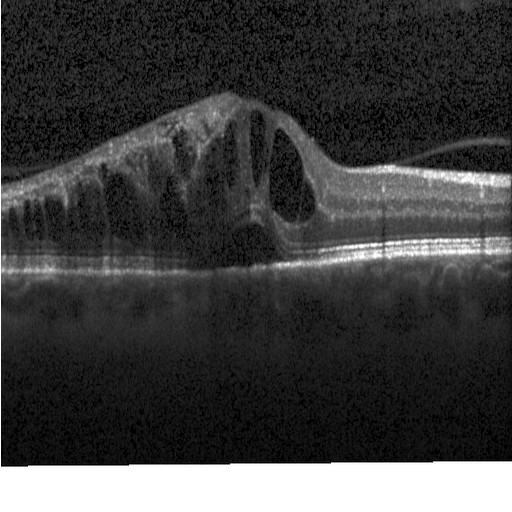

This B-scan demonstrates diabetic macular edema (DME).